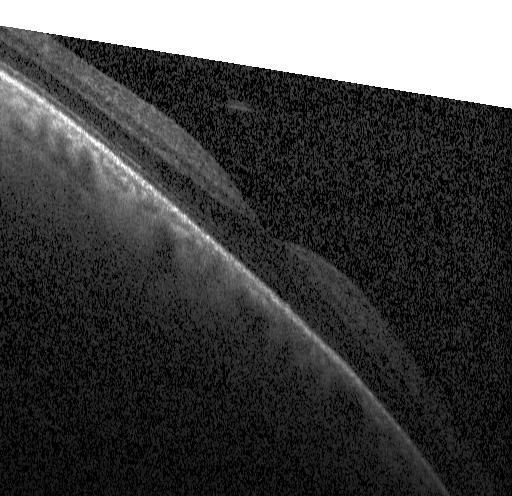 Retinal OCT cross-section showing neither choroidal neovascularization, diabetic macular edema, nor drusen.